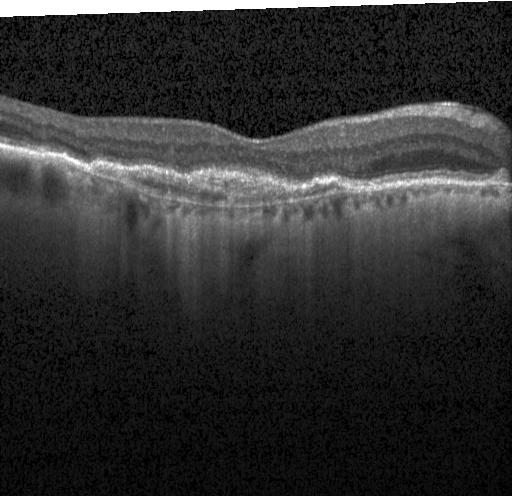 SD-OCT, retinal OCT B-scan.
OCT finding: choroidal neovascularization (CNV).